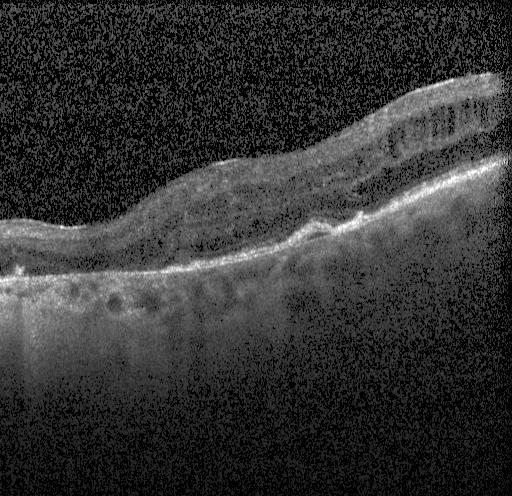

Impression: choroidal neovascularization.